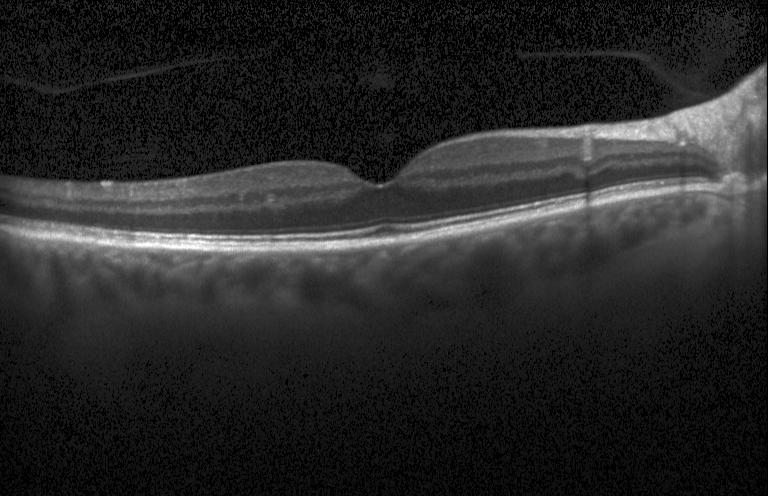

OCT line scan, macular scan, instrument: Heidelberg Spectralis, spectral-domain optical coherence tomography
Impression: no choroidal neovascularization, no diabetic macular edema, and no drusen.